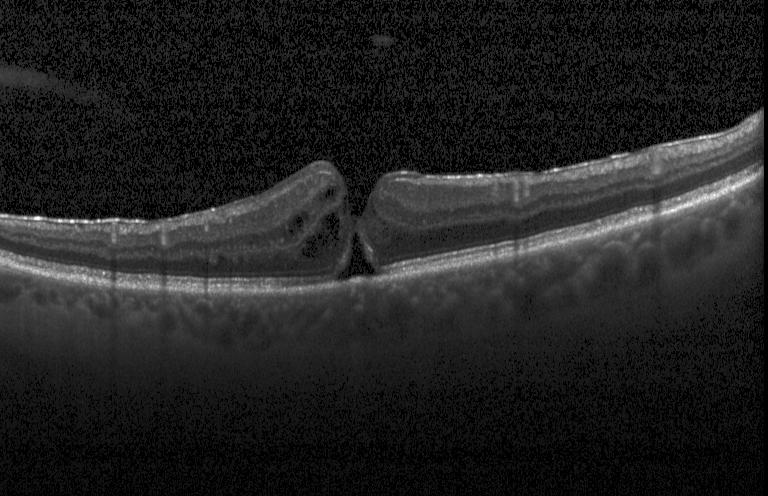 Heidelberg Spectralis. OCT line scan. Spectral-domain OCT. Through the macula — Diagnosis: diabetic macular edema (DME).